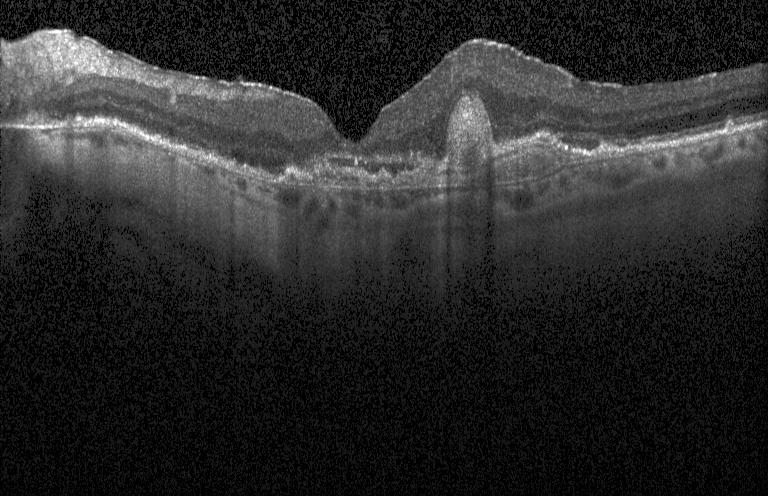 Acquired on a Heidelberg Spectralis, spectral-domain optical coherence tomography, optical coherence tomography scan
Finding: a choroidal neovascular membrane.